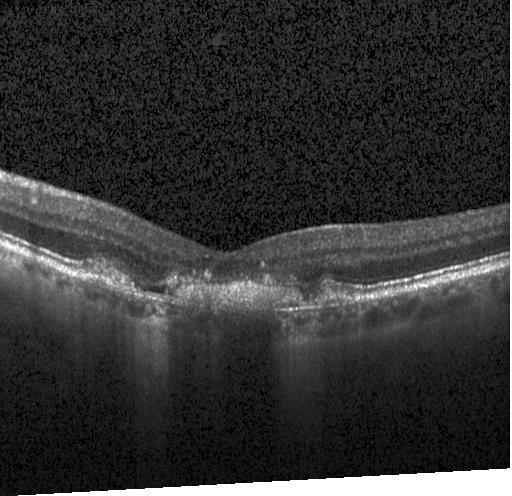
OCT scan showing a choroidal neovascular membrane.